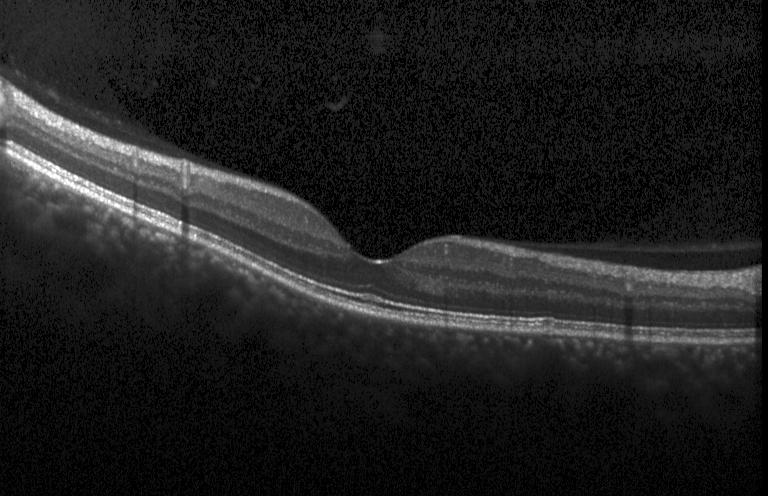
Heidelberg Spectralis · horizontal scan through the fovea · OCT line scan · spectral-domain optical coherence tomography.
This B-scan demonstrates no evidence of CNV, DME, or drusen.